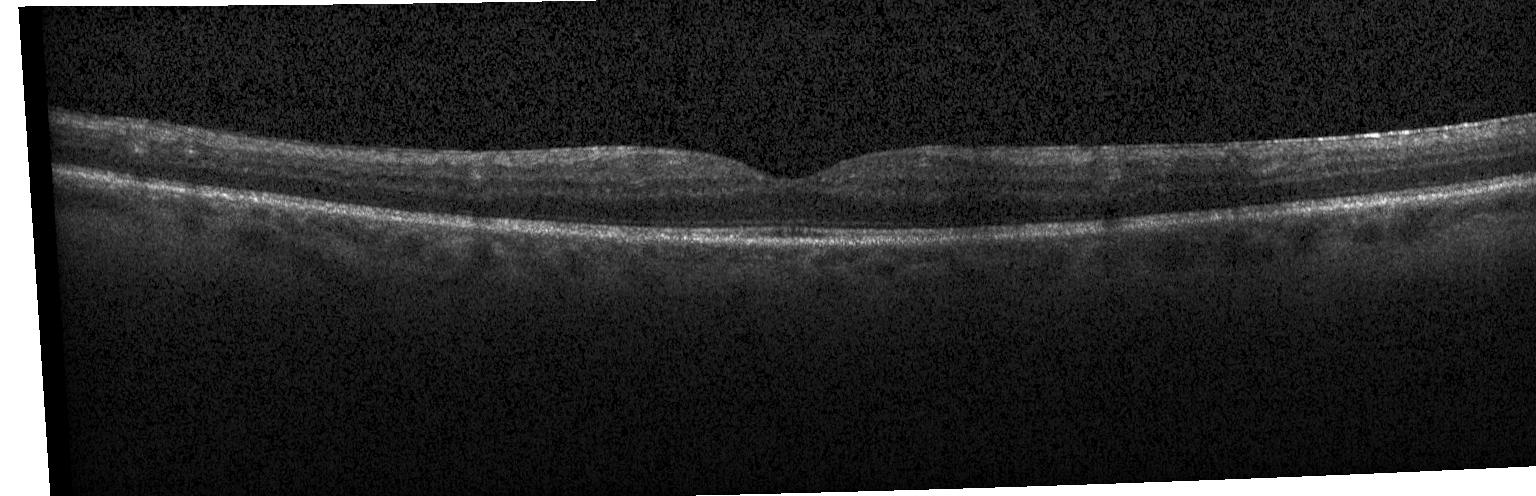

Impression: no evidence of choroidal neovascularization, diabetic macular edema, or drusen.